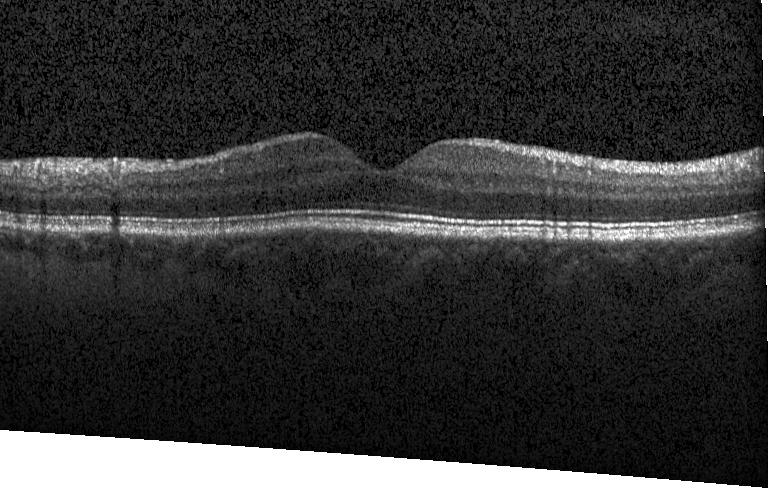
Centered on the fovea; OCT line scan
The scan shows no evidence of choroidal neovascularization, diabetic macular edema, or drusen.